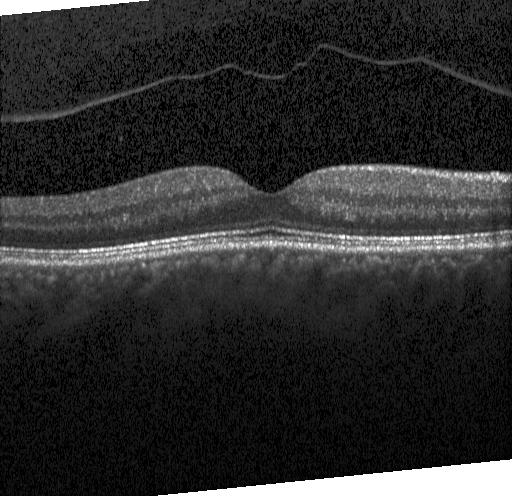

Macular OCT: neither choroidal neovascularization, diabetic macular edema, nor drusen.